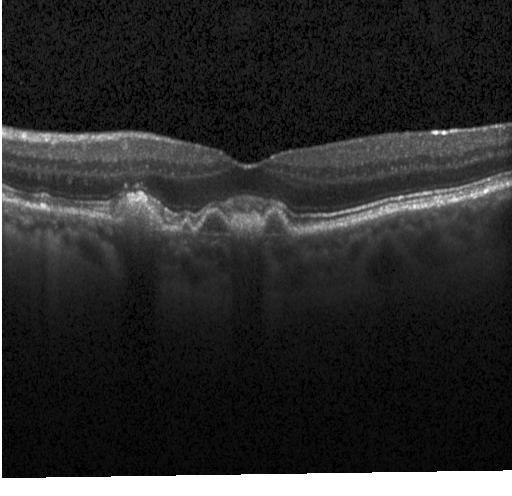
Retinal OCT B-scan; SD-OCT.
Impression: choroidal neovascularization.